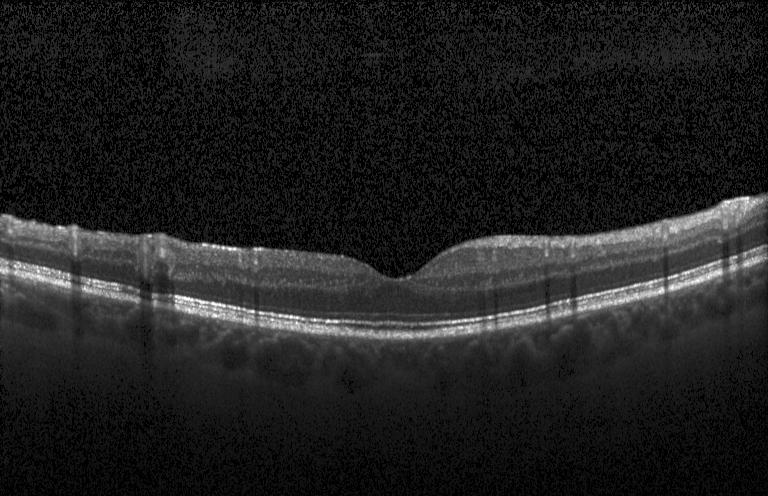

Finding: no evidence of choroidal neovascularization, diabetic macular edema, or drusen.